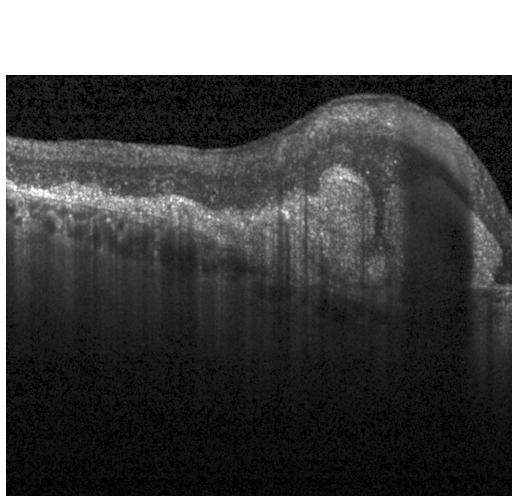

SD-OCT. Fovea-centered. Acquired on a Heidelberg Spectralis. Optical coherence tomography B-scan. Assessment: a choroidal neovascular membrane.